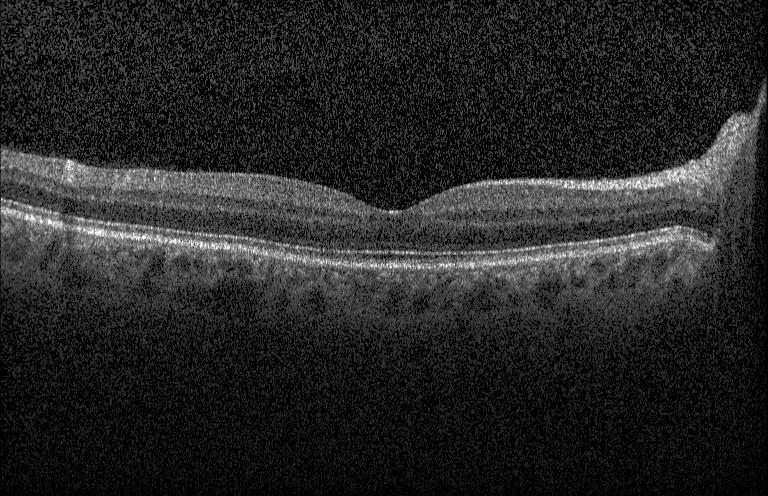

Impression: no CNV, DME, or drusen.